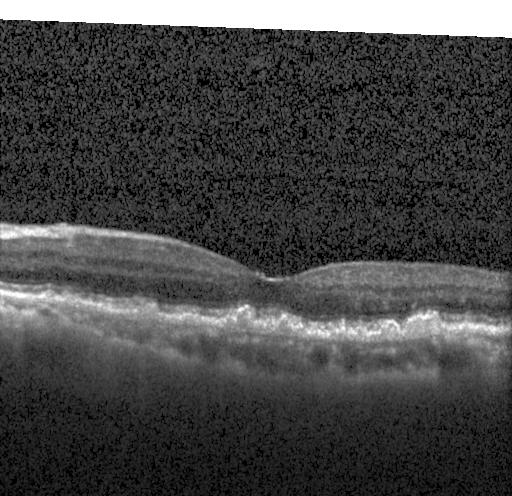 Heidelberg Spectralis. SD-OCT. Retinal OCT B-scan. Macular scan
Diagnosis: sub-RPE drusenoid deposits.